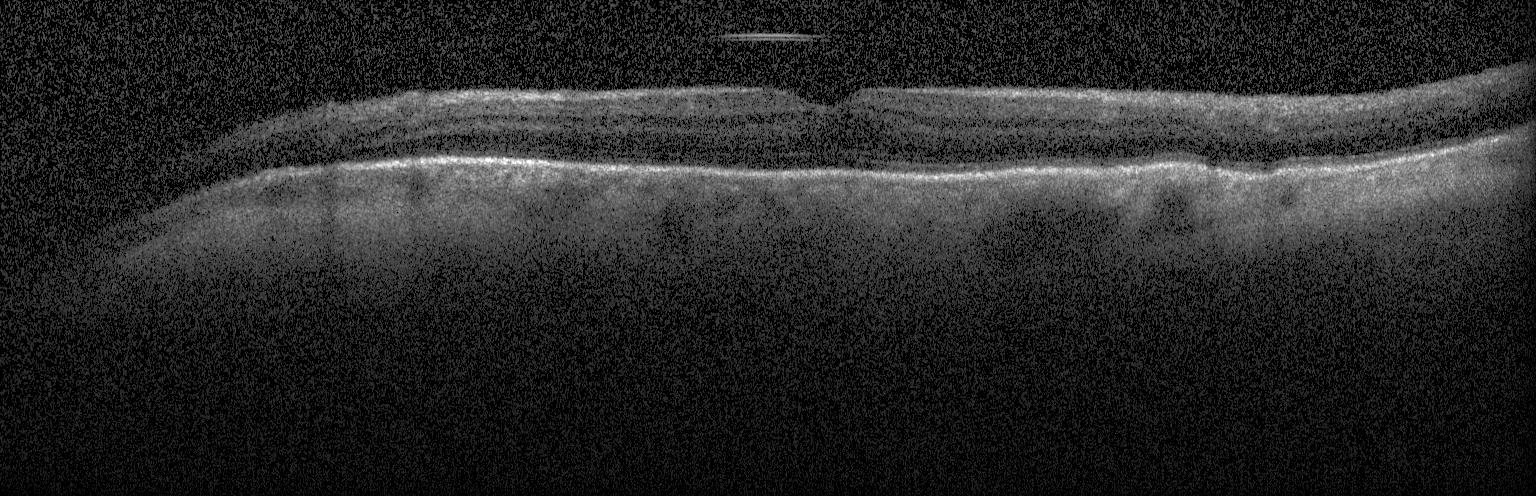
OCT line scan · centered on the fovea — Finding: no CNV, DME, or drusen.